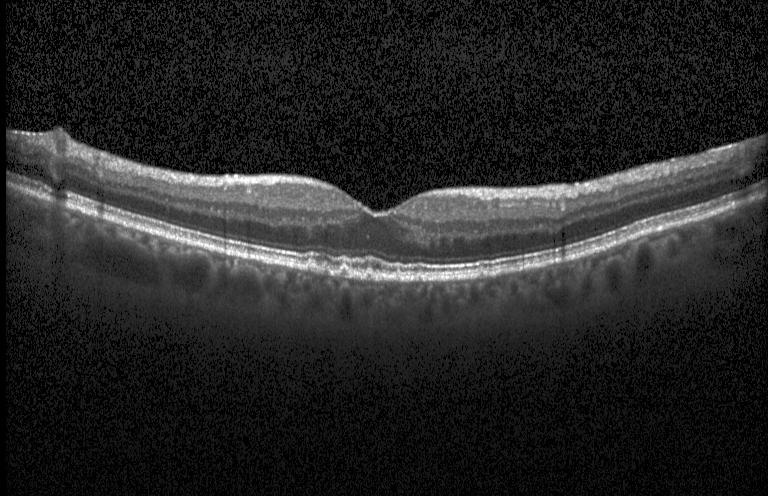 Optical coherence tomography B-scan — Impression: drusen.